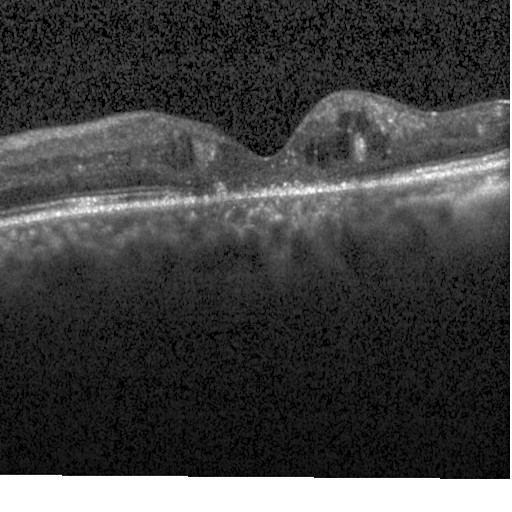
Retinal OCT B-scan. Fovea-centered. Spectral-domain OCT — OCT finding: diabetic macular edema.